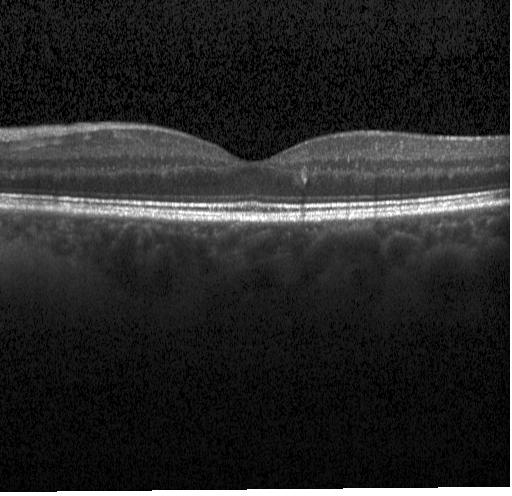

Centered on the fovea. Spectral-domain optical coherence tomography. Instrument: Heidelberg Spectralis. Optical coherence tomography scan. Dx: no CNV, no DME, and no drusen.